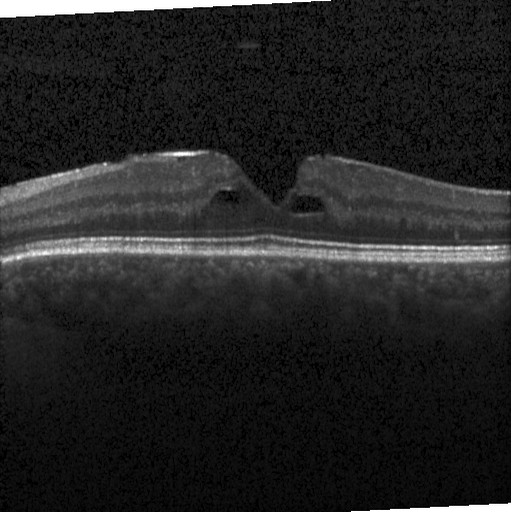

Finding: diabetic macular edema.